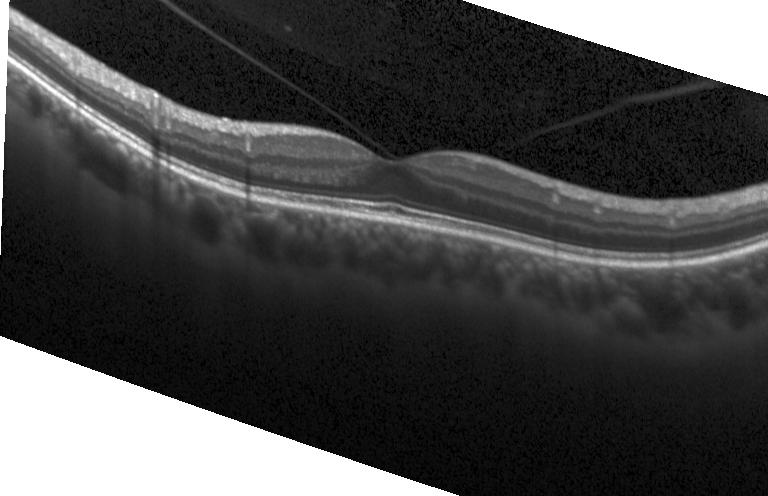

Centered on the fovea, optical coherence tomography B-scan, instrument: Heidelberg Spectralis — Dx: neither choroidal neovascularization, diabetic macular edema, nor drusen.